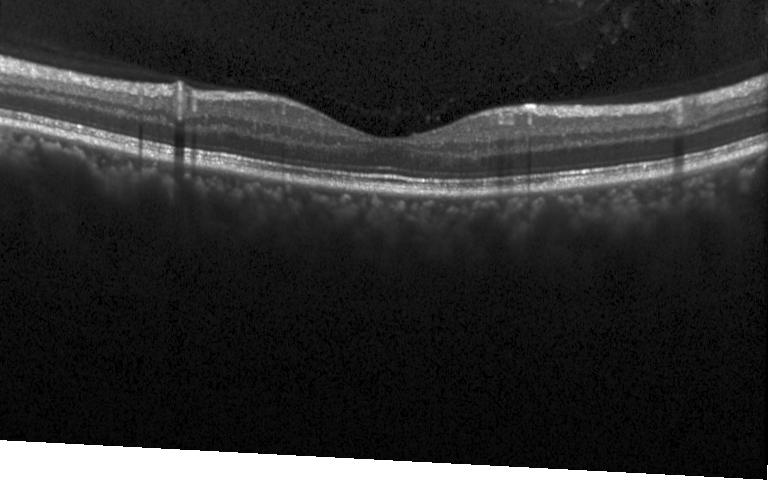 Fovea-centered, retinal OCT cross-section — Diagnosis: no evidence of choroidal neovascularization, diabetic macular edema, or drusen.